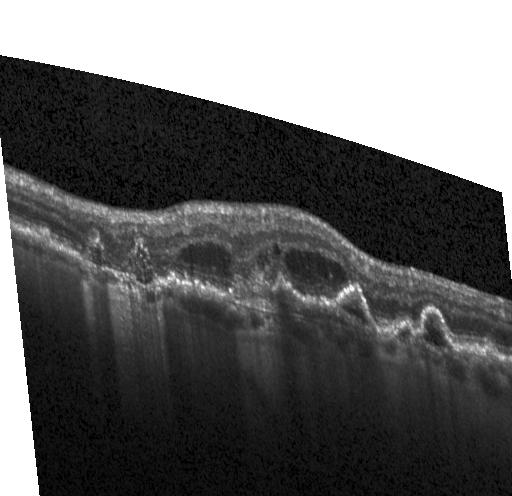
Optical coherence tomography B-scan
The scan shows choroidal neovascularization.